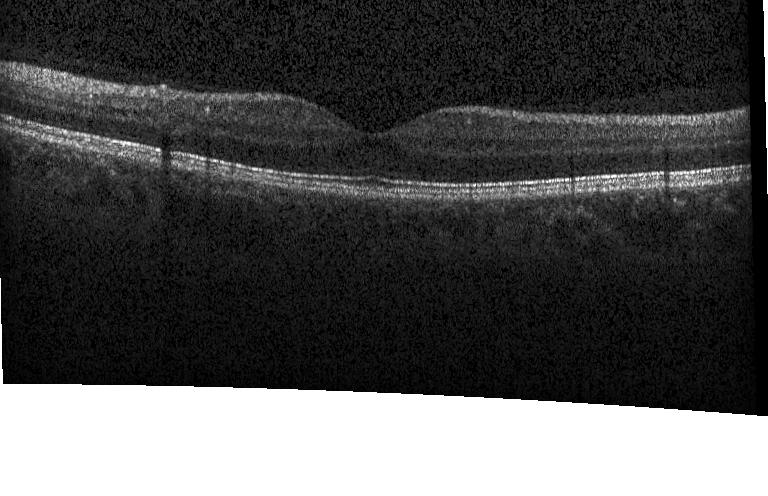
OCT B-scan showing no evidence of CNV, DME, or drusen.